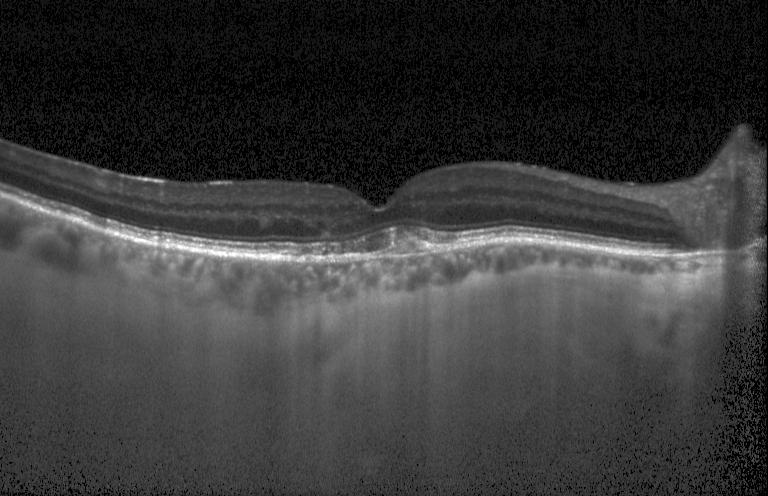 Dx: a choroidal neovascular membrane.